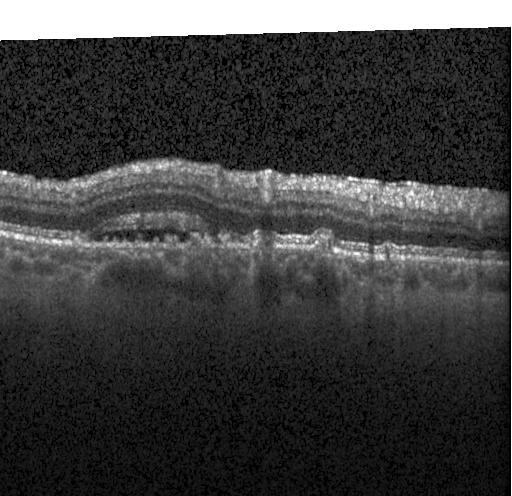

Macular OCT: choroidal neovascularization.